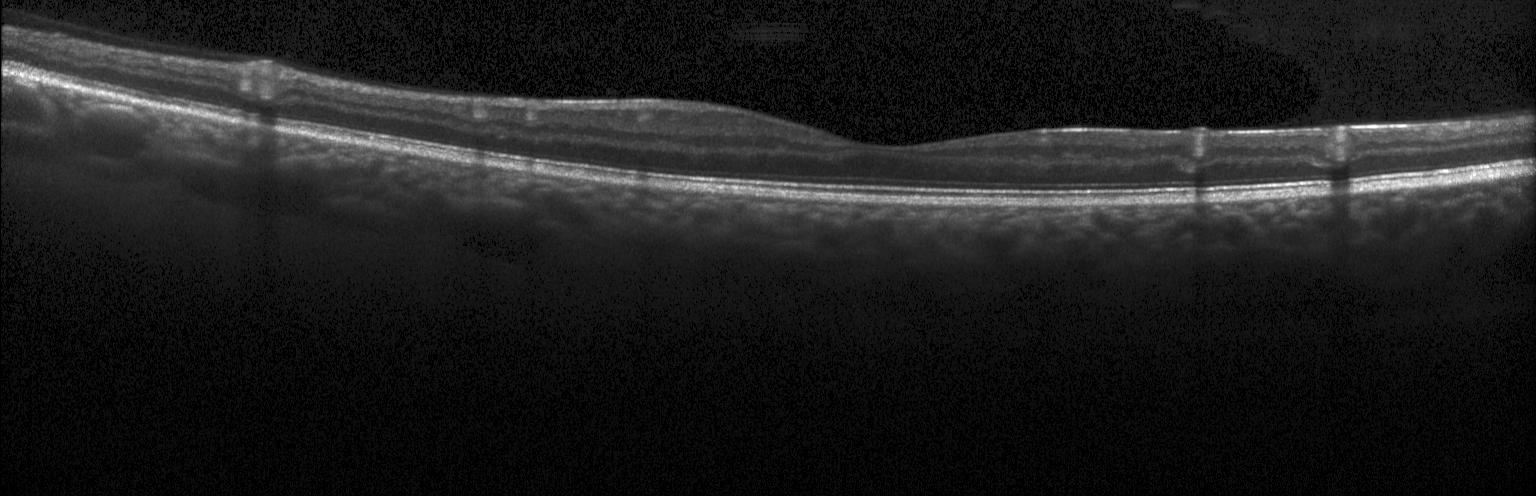 Diagnosis: neither CNV, DME, nor drusen.